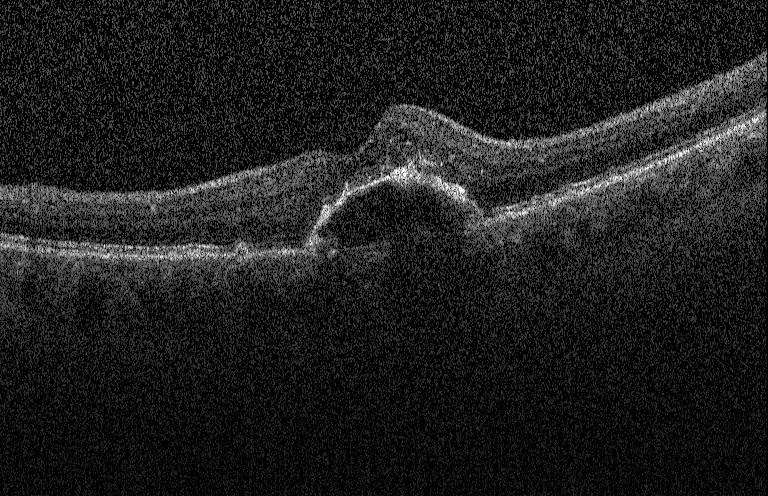
Optical coherence tomography scan — Choroidal neovascularization.